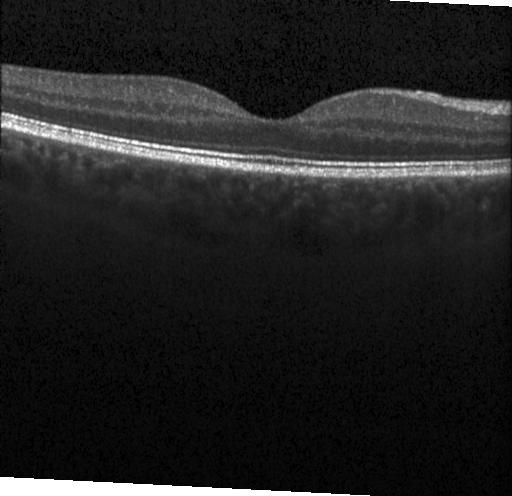

OCT B-scan. Macular OCT: no evidence of choroidal neovascularization, diabetic macular edema, or drusen.